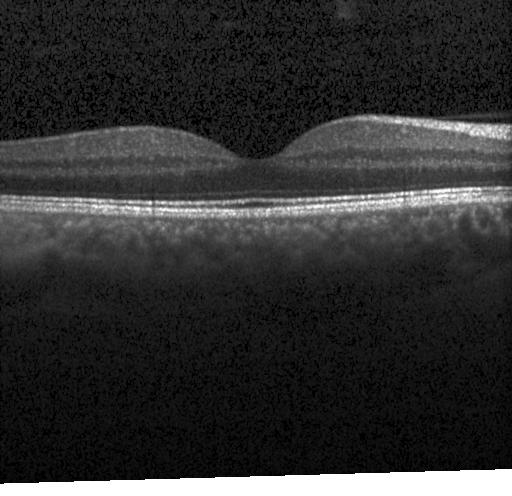
Macular OCT demonstrating no CNV, DME, or drusen.